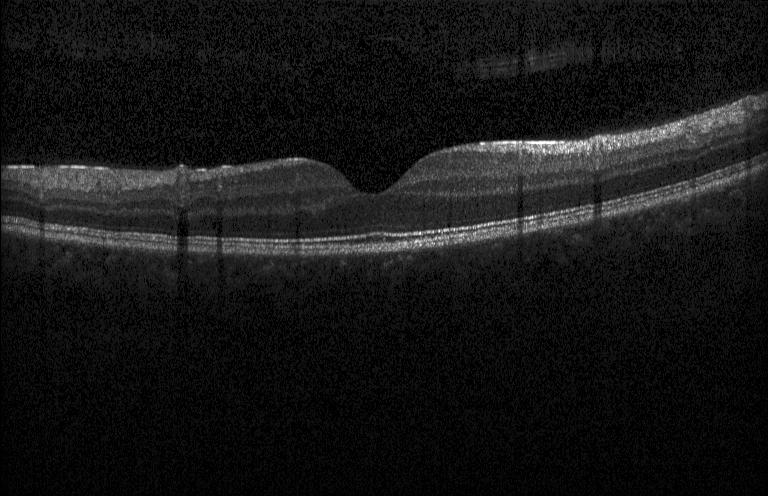
Optical coherence tomography scan · SD-OCT · Heidelberg Spectralis — Diagnosis: neither choroidal neovascularization, diabetic macular edema, nor drusen.